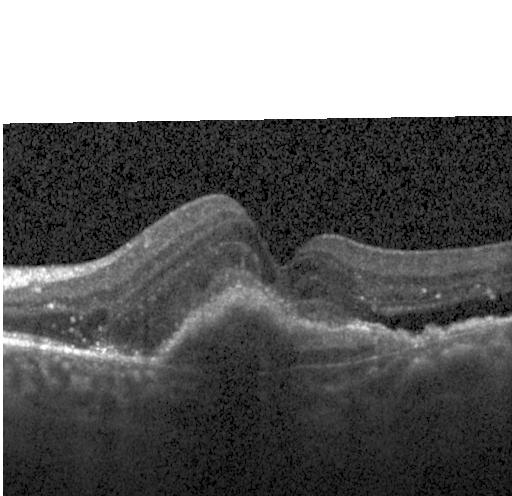

Through the macula. SD-OCT. Optical coherence tomography scan. Instrument: Heidelberg Spectralis.
Macular OCT: choroidal neovascularization.